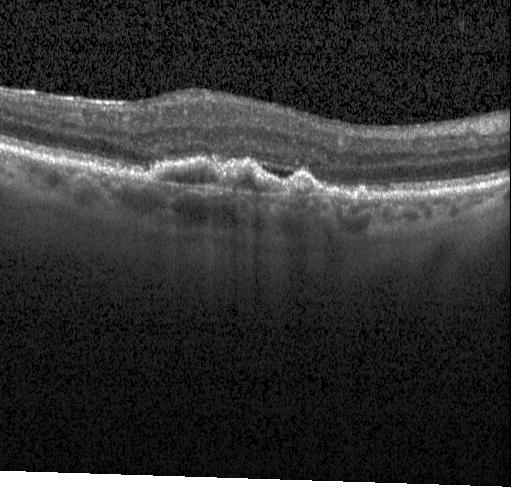 Fovea-centered · instrument: Heidelberg Spectralis · retinal OCT cross-section · spectral-domain OCT
Impression: choroidal neovascularization.